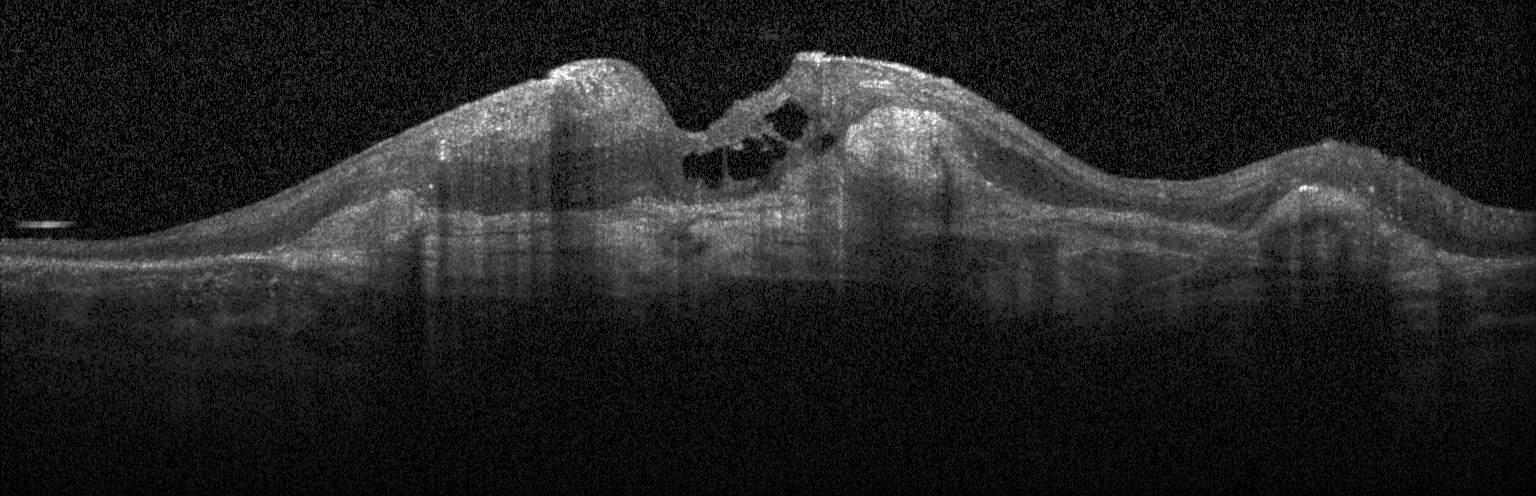

Impression: CNV.